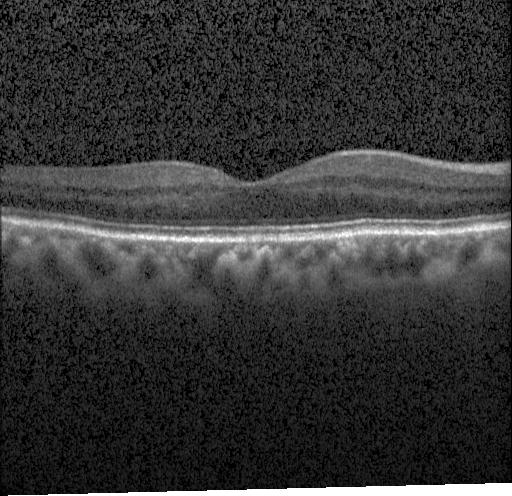 OCT line scan, spectral-domain OCT, horizontal scan through the fovea, acquired on a Heidelberg Spectralis.
Impression: no CNV, no DME, and no drusen.